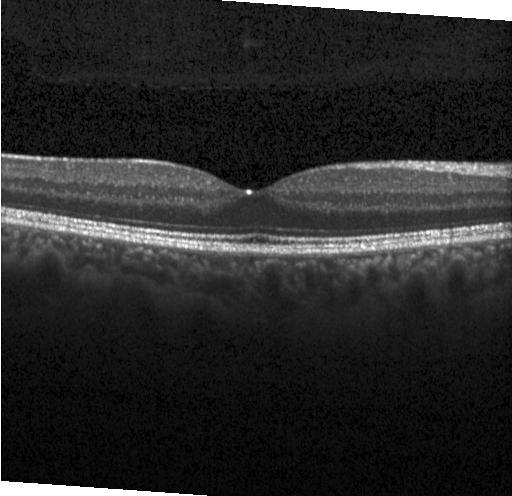
OCT B-scan
OCT finding: no choroidal neovascularization, no diabetic macular edema, and no drusen.